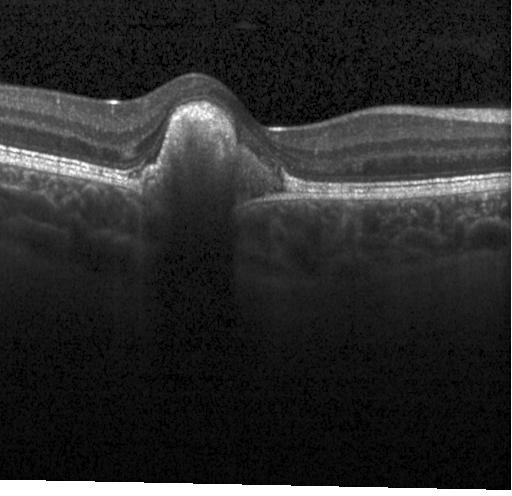 Through the macula, OCT B-scan — OCT finding: choroidal neovascularization (CNV).